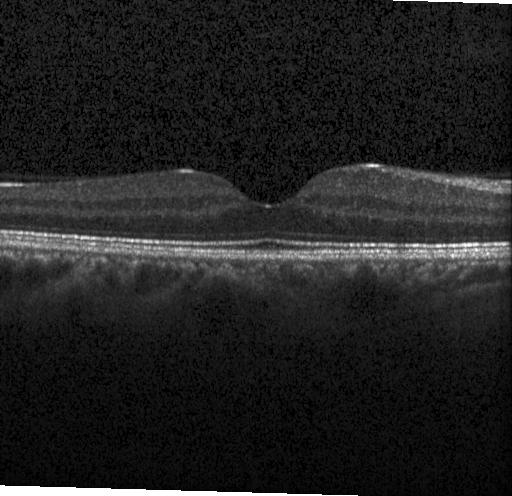

Impression: no choroidal neovascularization, no diabetic macular edema, and no drusen.